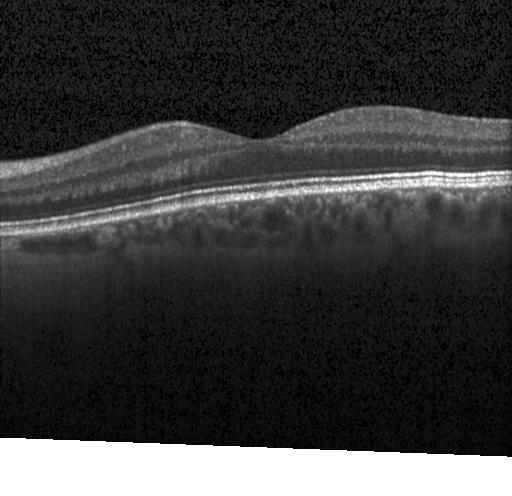 OCT finding: neither choroidal neovascularization, diabetic macular edema, nor drusen.